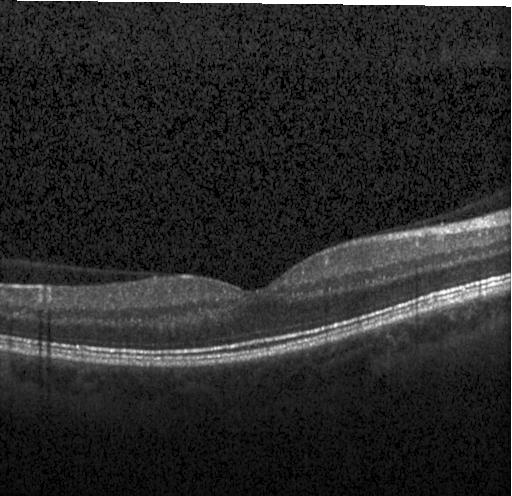 This B-scan demonstrates no choroidal neovascularization, no diabetic macular edema, and no drusen.